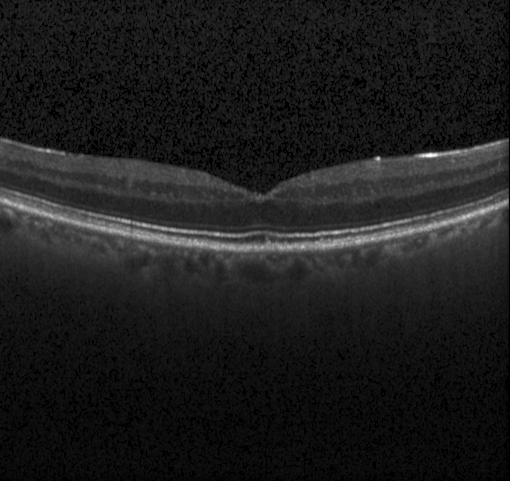
Spectral-domain OCT; Heidelberg Spectralis; macular scan; retinal OCT cross-section — This B-scan demonstrates no choroidal neovascularization, no diabetic macular edema, and no drusen.